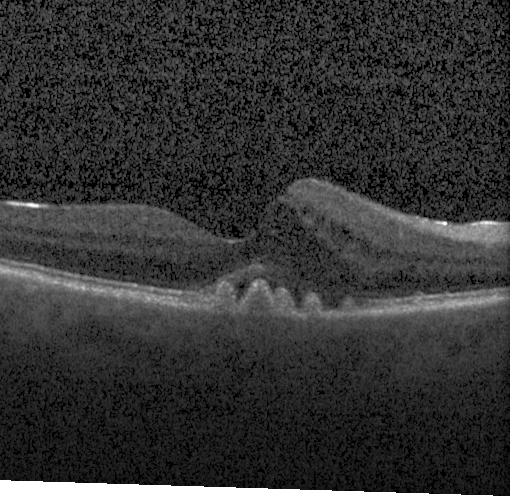

OCT B-scan · centered on the fovea.
OCT finding: a choroidal neovascular membrane.